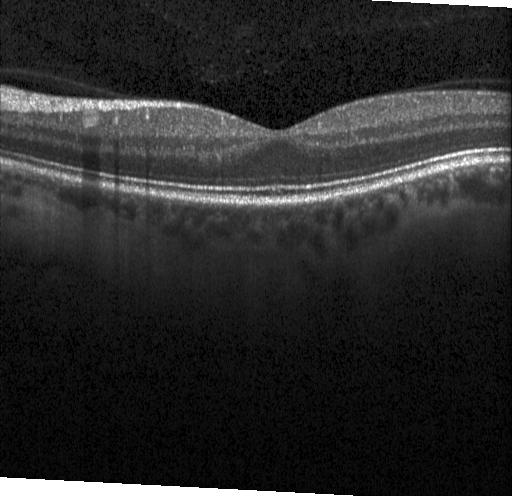

Spectral-domain OCT · retinal OCT cross-section · macular scan
Diagnosis: no choroidal neovascularization, diabetic macular edema, or drusen.